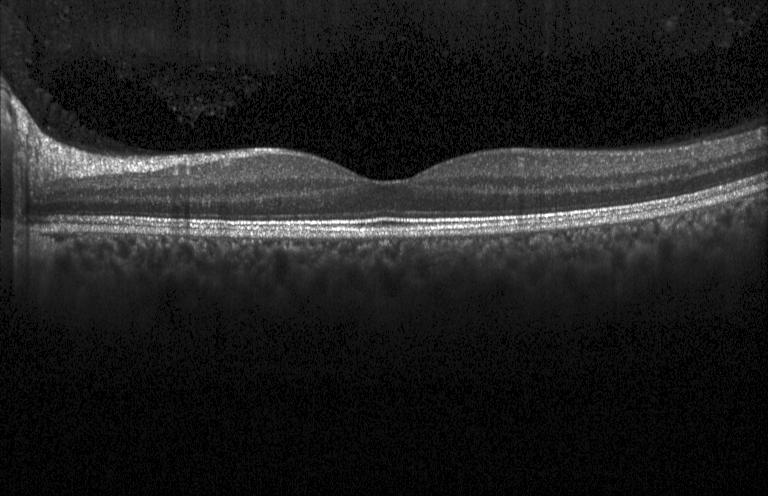
Heidelberg Spectralis OCT system. Optical coherence tomography B-scan. Diagnosis: no choroidal neovascularization, diabetic macular edema, or drusen.